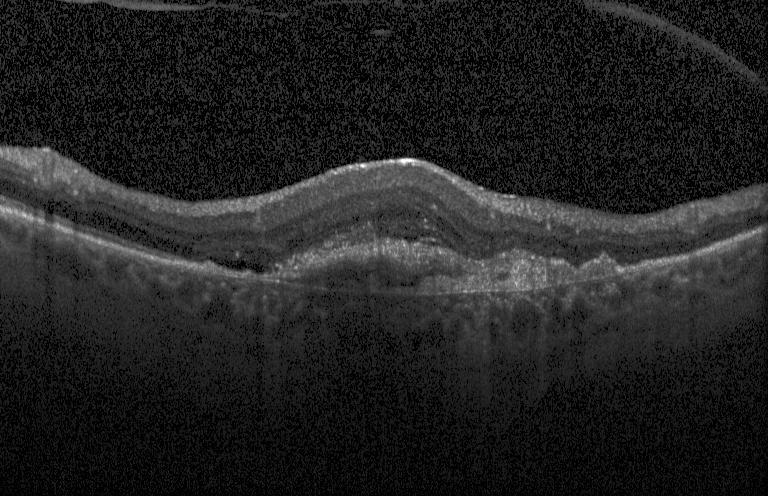

Centered on the fovea. Retinal OCT B-scan. Heidelberg Spectralis. SD-OCT
This B-scan demonstrates choroidal neovascularization.